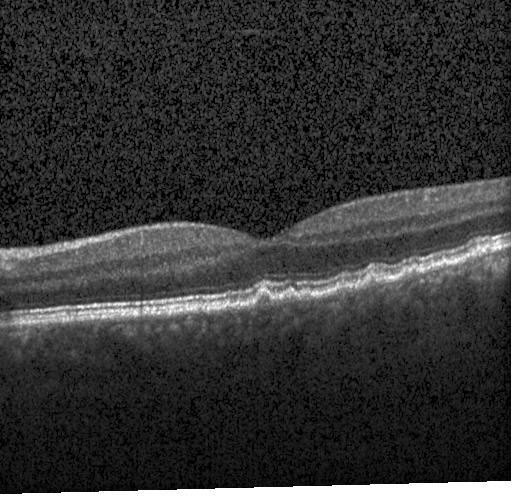

Finding: drusen.